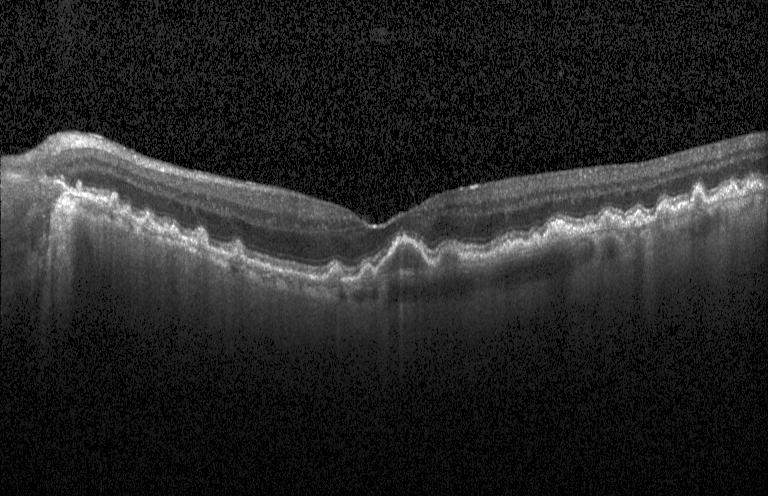

Retinal OCT B-scan
This B-scan demonstrates sub-RPE drusenoid deposits.